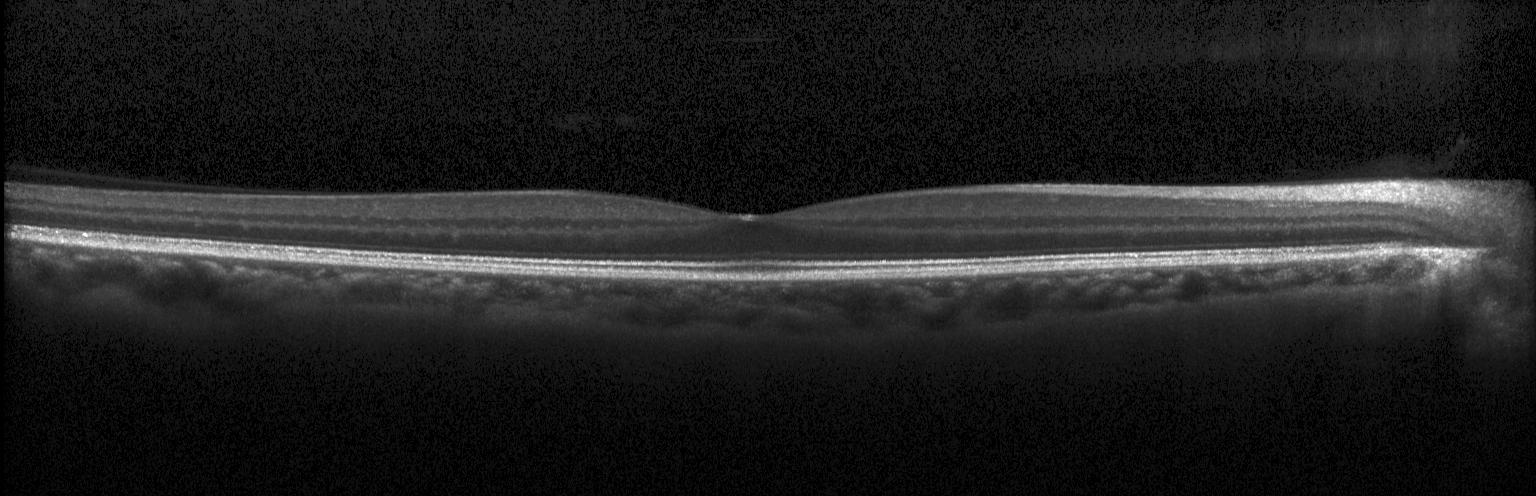

Diagnosis: neither choroidal neovascularization, diabetic macular edema, nor drusen.